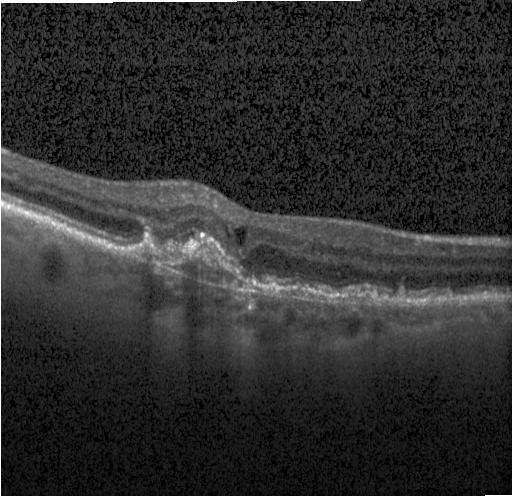
Spectral-domain OCT B-scan: choroidal neovascularization.